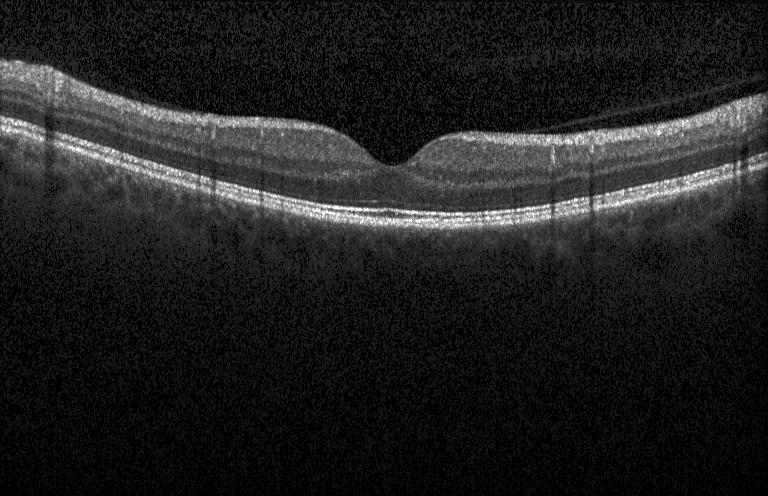 Optical coherence tomography B-scan — Impression: no choroidal neovascularization, no diabetic macular edema, and no drusen.